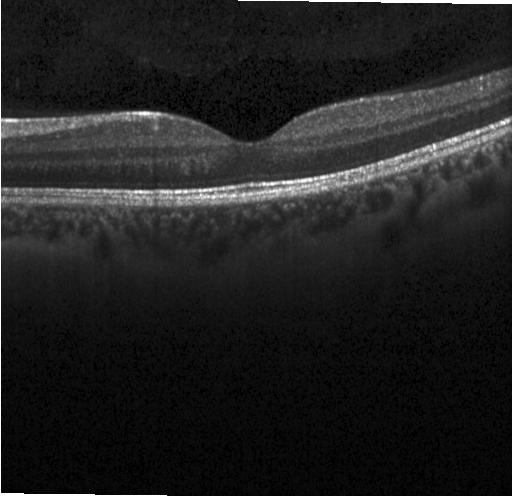 Optical coherence tomography B-scan, Heidelberg Spectralis, fovea-centered
No evidence of choroidal neovascularization, diabetic macular edema, or drusen.